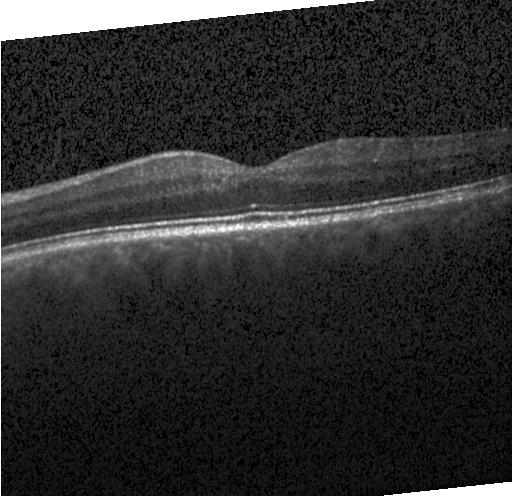
Assessment: neither CNV, DME, nor drusen.